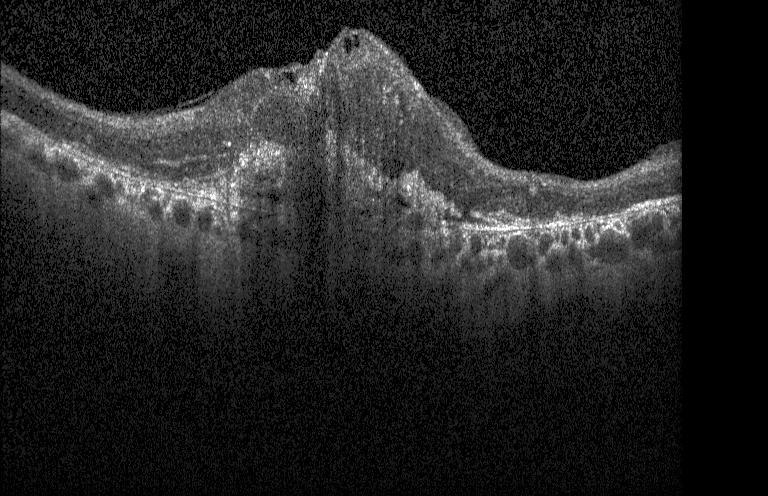 Spectral-domain optical coherence tomography, OCT line scan. A choroidal neovascular membrane.